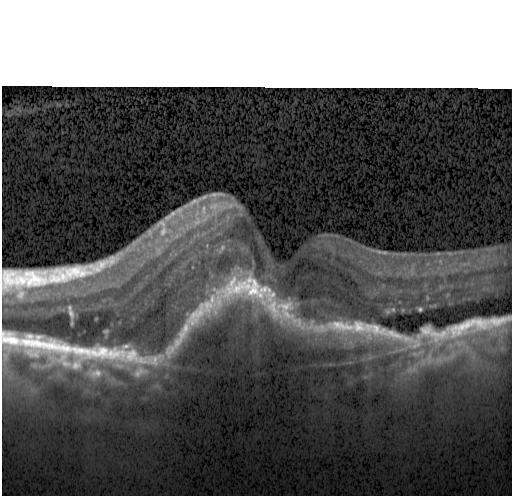
Optical coherence tomography B-scan — Impression: CNV.